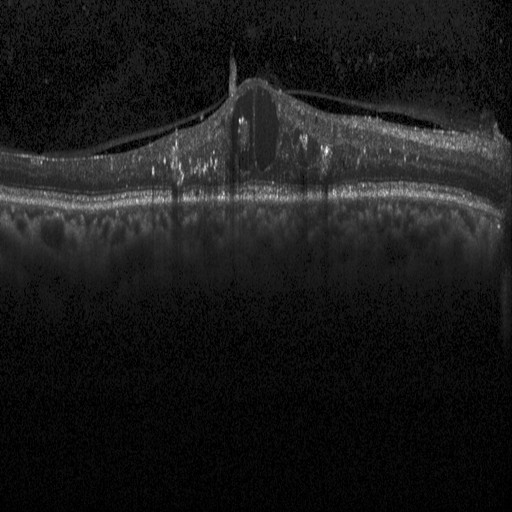
OCT B-scan. Horizontal scan through the fovea. Heidelberg Spectralis — Assessment: diabetic macular edema (DME).